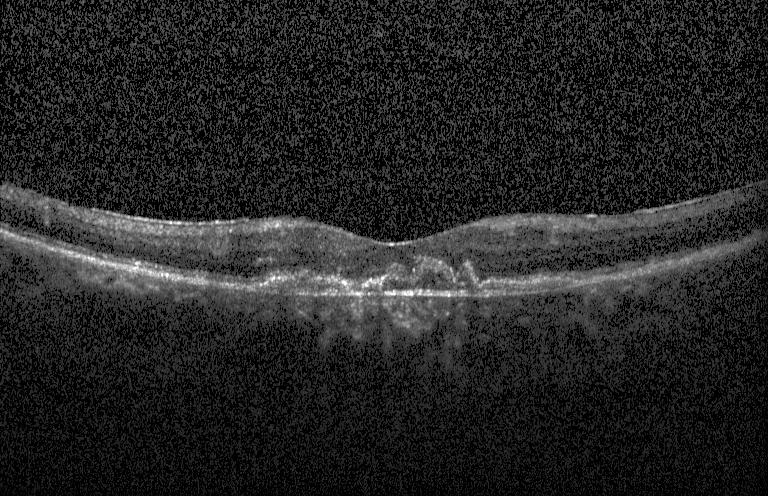 OCT line scan.
The scan shows CNV.